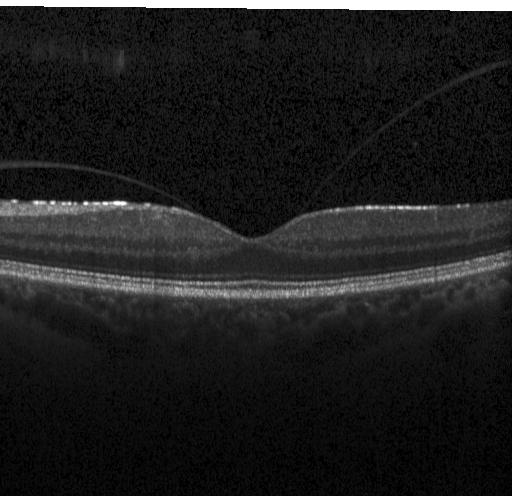

Retinal OCT cross-section.
Diagnosis: no choroidal neovascularization, diabetic macular edema, or drusen.